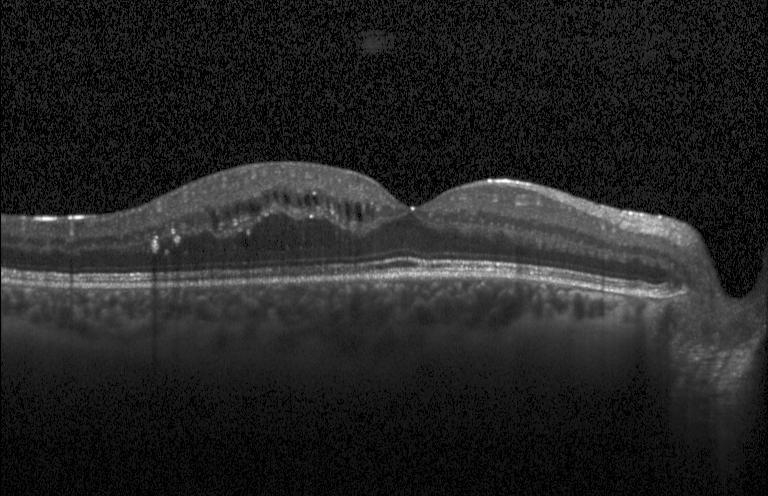

DME.